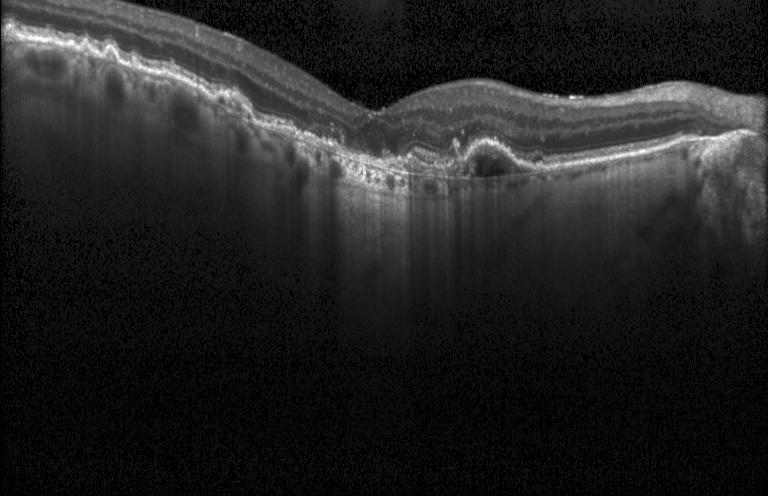

SD-OCT · macular scan · OCT line scan · instrument: Heidelberg Spectralis. Finding: a choroidal neovascular membrane.